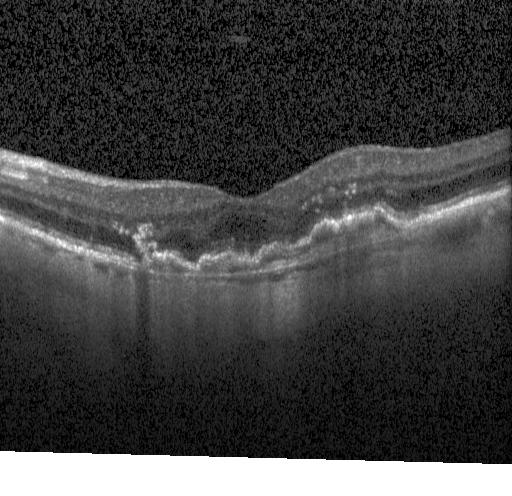 Retinal OCT cross-section showing choroidal neovascularization (CNV).